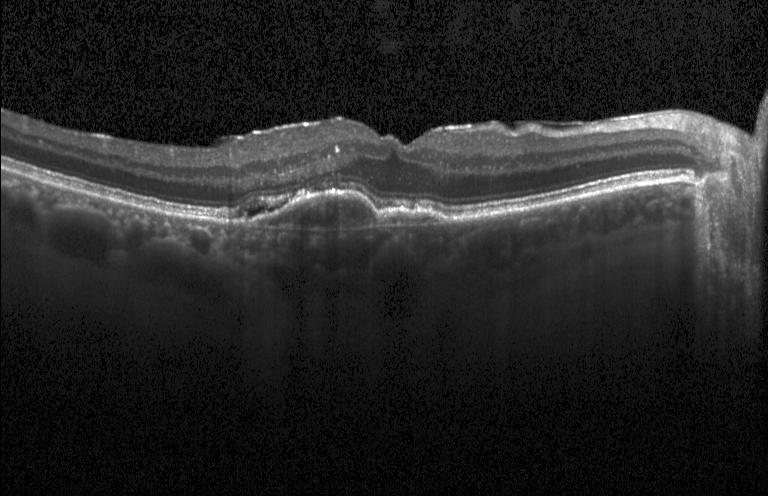
Finding: choroidal neovascularization (CNV).